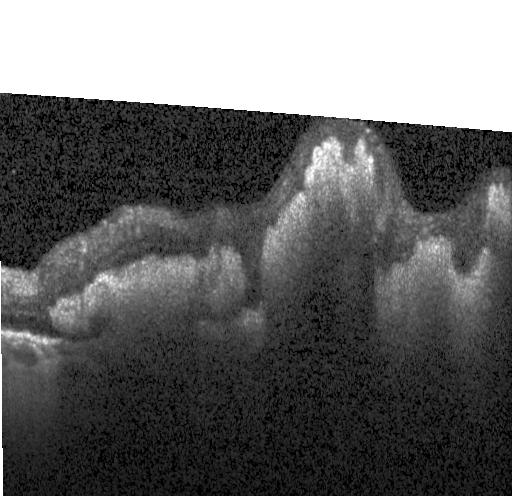

SD-OCT · retinal OCT B-scan · fovea-centered · acquired on a Heidelberg Spectralis — Diagnosis: choroidal neovascularization.